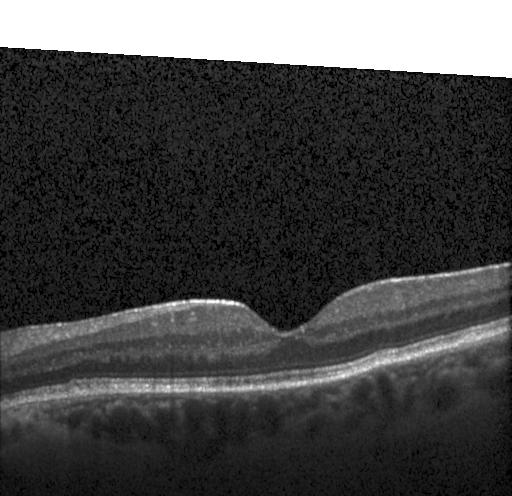
No choroidal neovascularization, diabetic macular edema, or drusen.